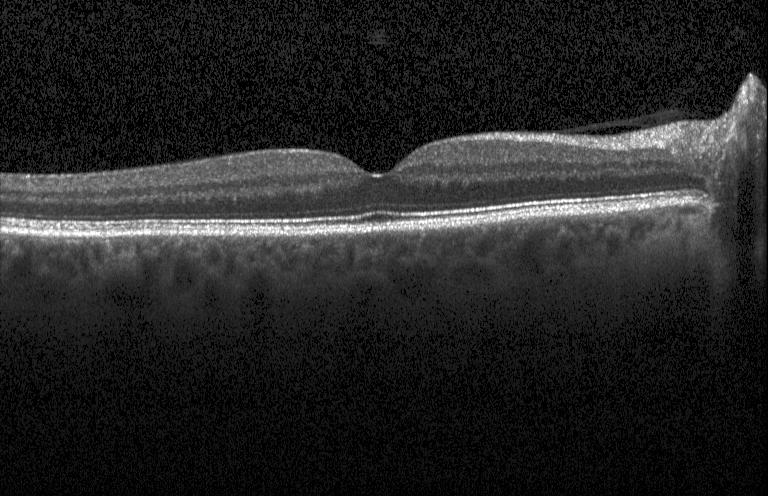

Assessment: neither choroidal neovascularization, diabetic macular edema, nor drusen.